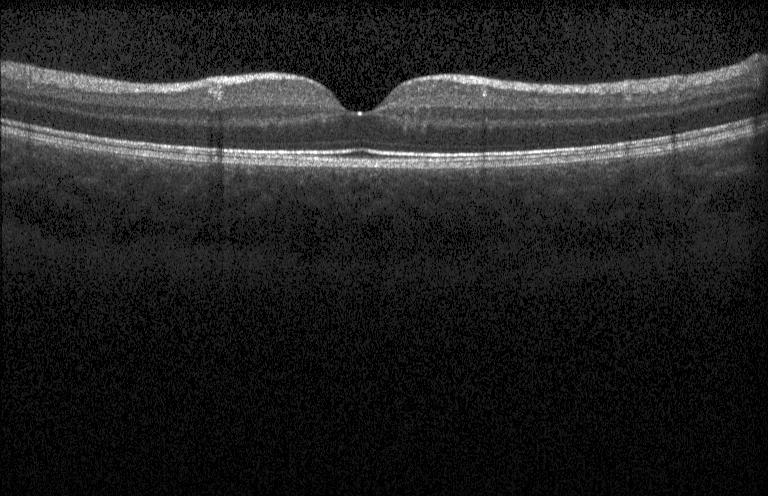

Finding: neither choroidal neovascularization, diabetic macular edema, nor drusen.